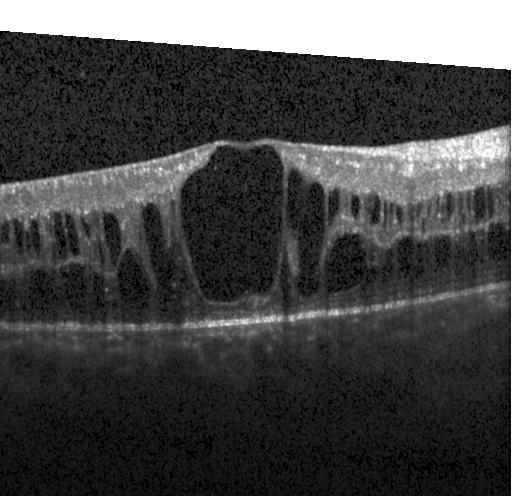

Macular OCT: diabetic macular edema (DME).